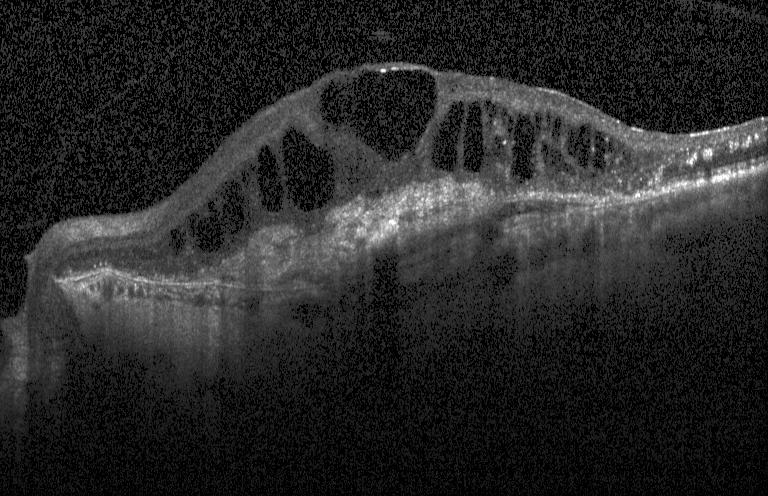
Horizontal scan through the fovea; Heidelberg Spectralis; SD-OCT; retinal OCT B-scan
Finding: a choroidal neovascular membrane.